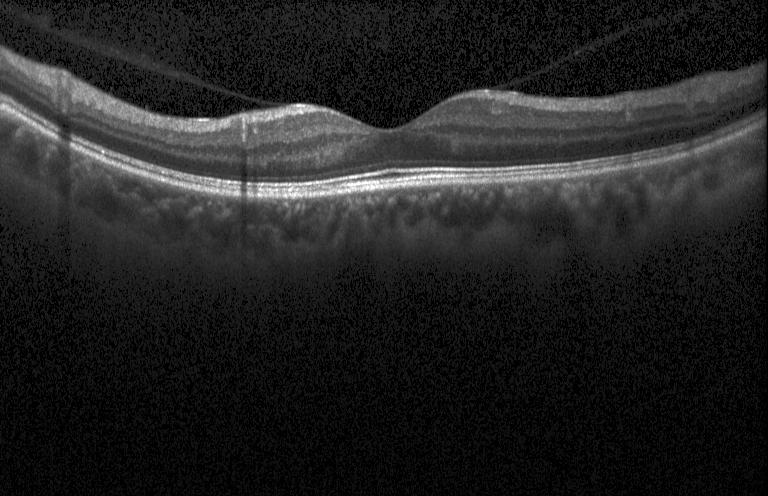 Horizontal scan through the fovea; retinal OCT cross-section; SD-OCT — OCT finding: no CNV, DME, or drusen.